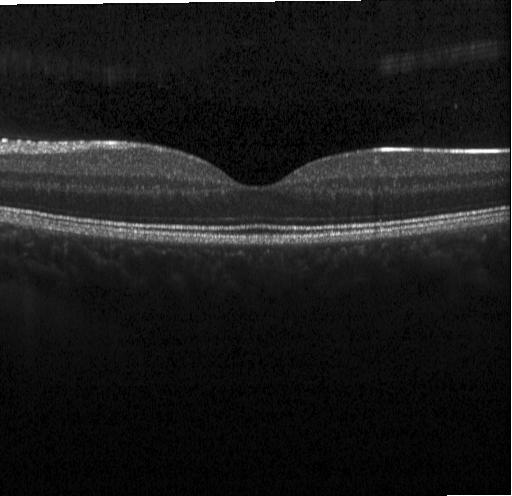
Acquired on a Heidelberg Spectralis · optical coherence tomography scan · SD-OCT · centered on the fovea — Impression: no choroidal neovascularization, no diabetic macular edema, and no drusen.